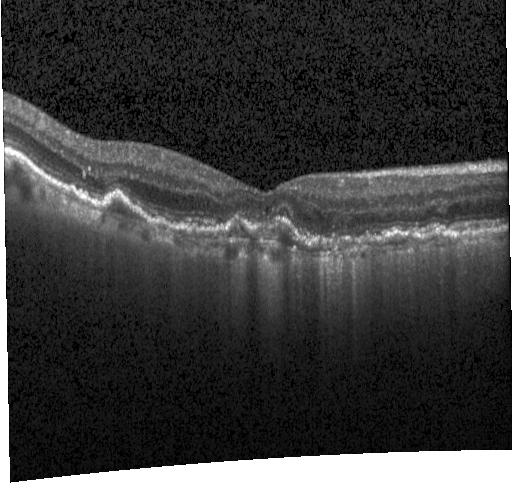 OCT line scan. Finding: a choroidal neovascular membrane.